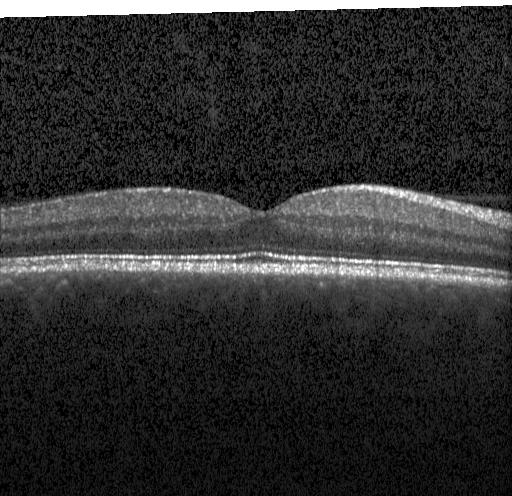

OCT B-scan — Diagnosis: no choroidal neovascularization, no diabetic macular edema, and no drusen.